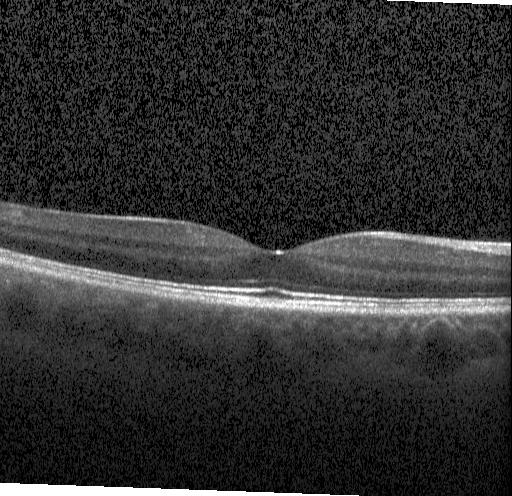 Spectral-domain OCT, optical coherence tomography scan, Heidelberg Spectralis OCT system, fovea-centered
Impression: no CNV, DME, or drusen.